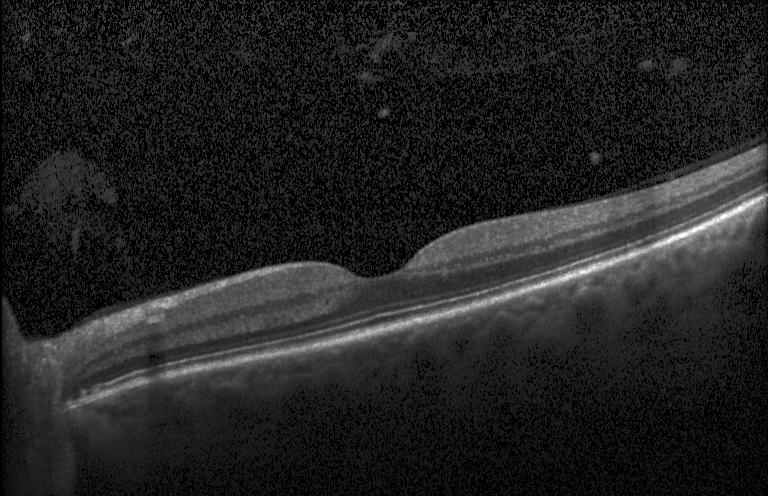
Acquired on a Heidelberg Spectralis, OCT B-scan. This B-scan demonstrates neither CNV, DME, nor drusen.